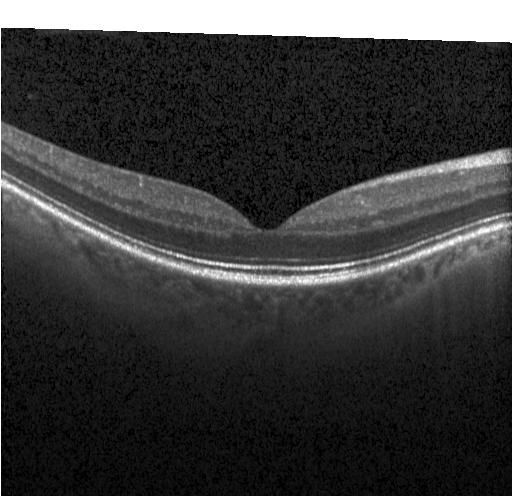

The scan shows no CNV, no DME, and no drusen.